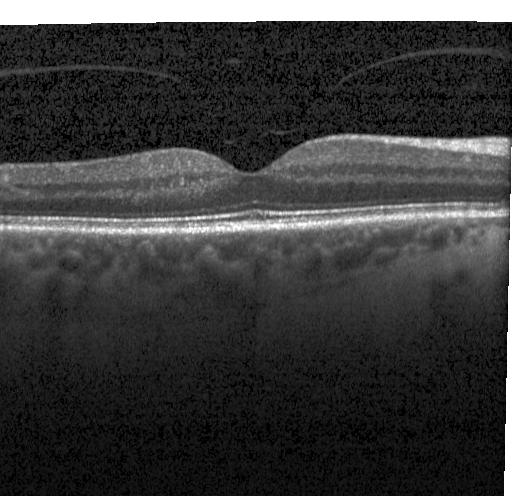
Macular OCT: no evidence of choroidal neovascularization, diabetic macular edema, or drusen.